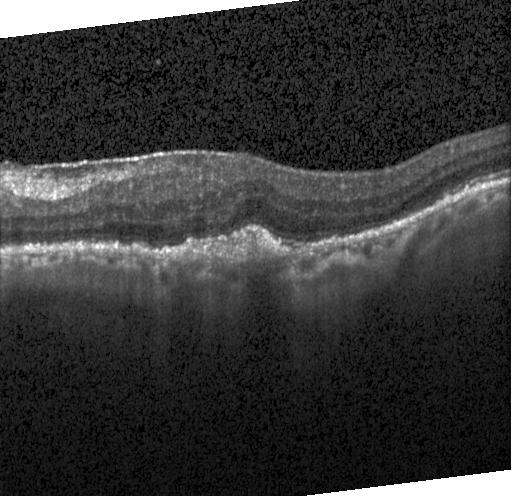 OCT scan showing choroidal neovascularization.